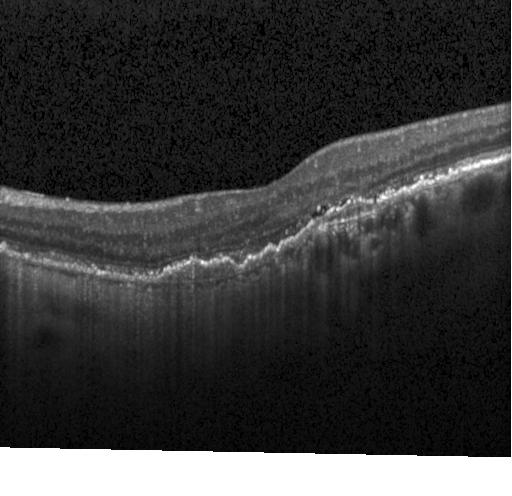 Optical coherence tomography scan; instrument: Heidelberg Spectralis.
Finding: a choroidal neovascular membrane.